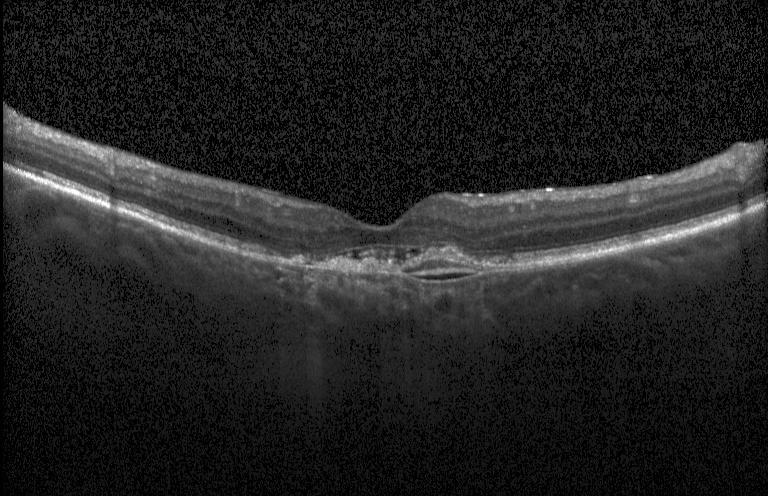

Optical coherence tomography B-scan. Diagnosis: CNV.